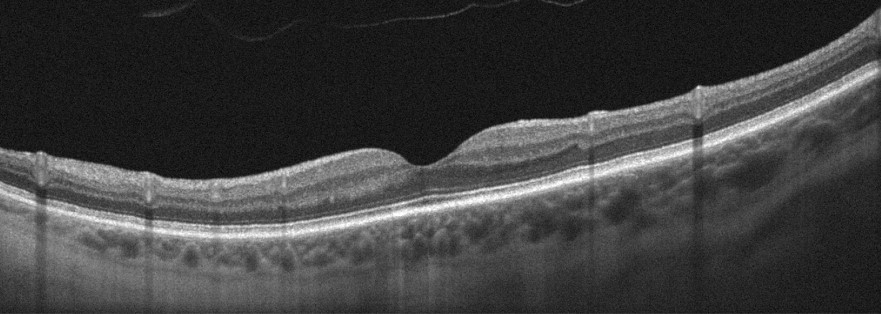

OCT line scan, instrument: Optovue Avanti RTVue XR, fovea-centered — Diagnosis: absence of AMD, DME, ERM, RAO, RVO, and vitreomacular interface disease.